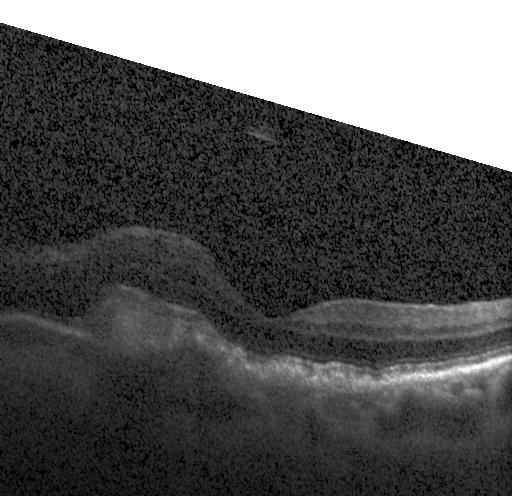 Assessment: CNV.